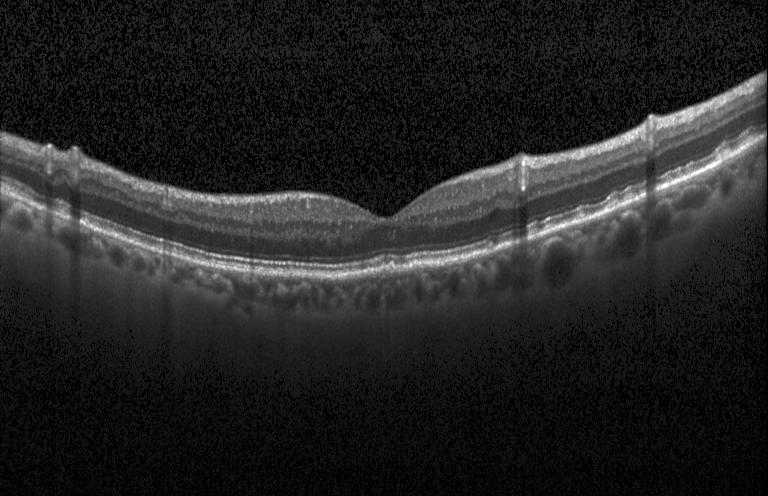

This B-scan demonstrates no choroidal neovascularization, no diabetic macular edema, and no drusen.